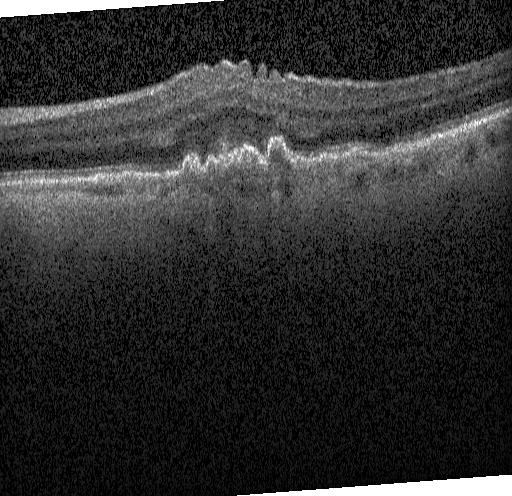 Retinal OCT cross-section showing CNV.